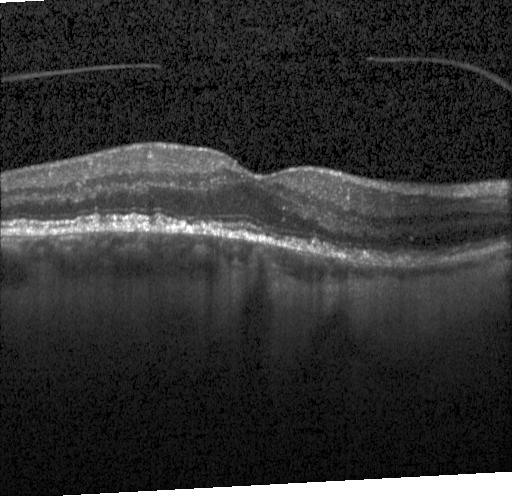

Retinal OCT cross-section — Impression: multiple drusen.